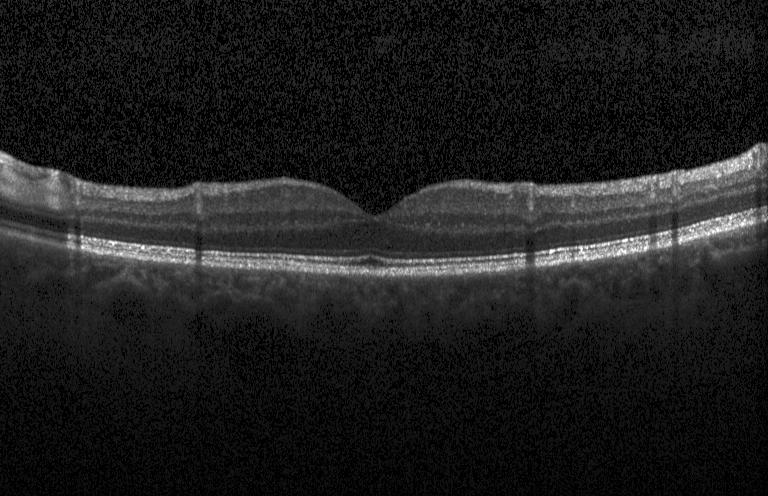
OCT line scan. Spectral-domain optical coherence tomography. Heidelberg Spectralis. Centered on the fovea
OCT finding: no evidence of choroidal neovascularization, diabetic macular edema, or drusen.